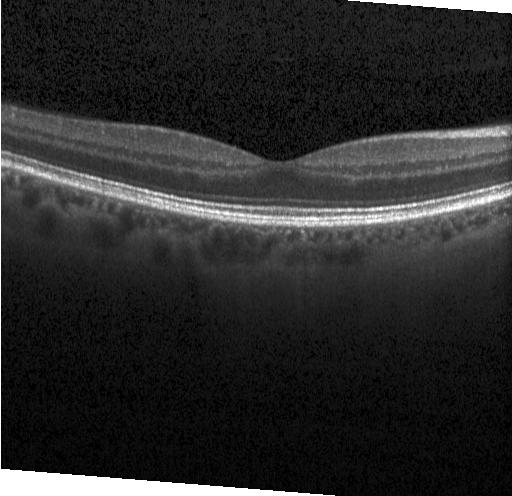 Retinal OCT cross-section — Finding: no choroidal neovascularization, no diabetic macular edema, and no drusen.